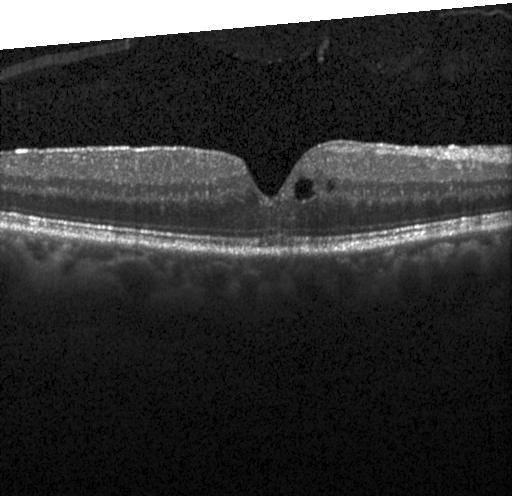 Fovea-centered, optical coherence tomography B-scan — Macular OCT: DME.